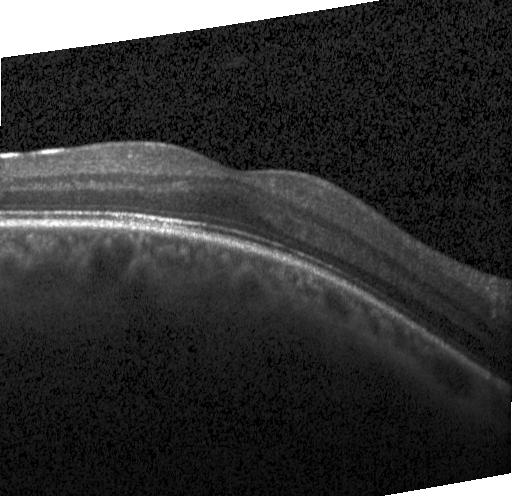

Optical coherence tomography scan; fovea-centered; spectral-domain OCT; acquired on a Heidelberg Spectralis.
The scan shows no choroidal neovascularization, no diabetic macular edema, and no drusen.